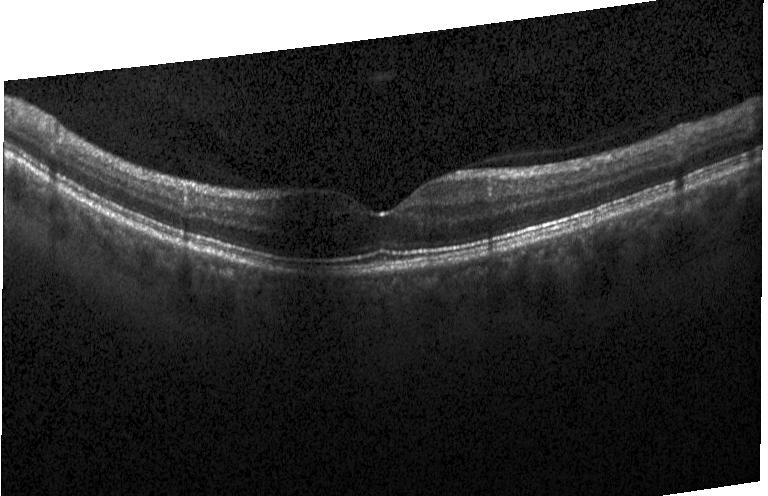
Centered on the fovea. Heidelberg Spectralis. SD-OCT. Optical coherence tomography B-scan. Finding: no choroidal neovascularization, no diabetic macular edema, and no drusen.